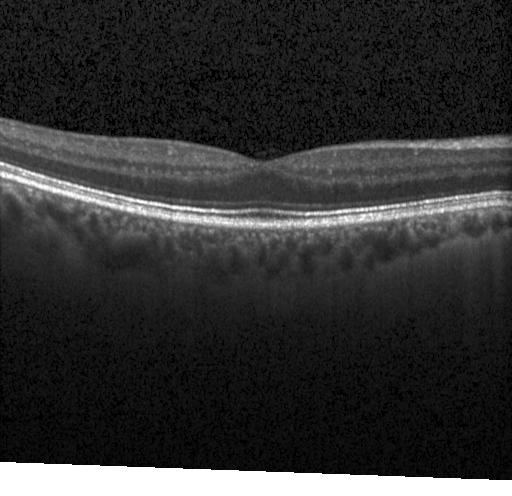

Assessment: no evidence of choroidal neovascularization, diabetic macular edema, or drusen.